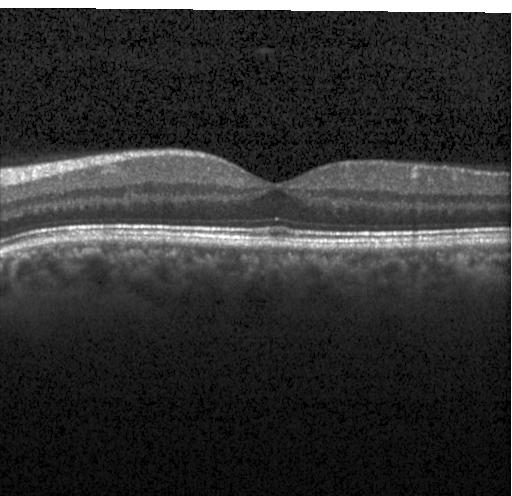
Macular OCT demonstrating no evidence of choroidal neovascularization, diabetic macular edema, or drusen.